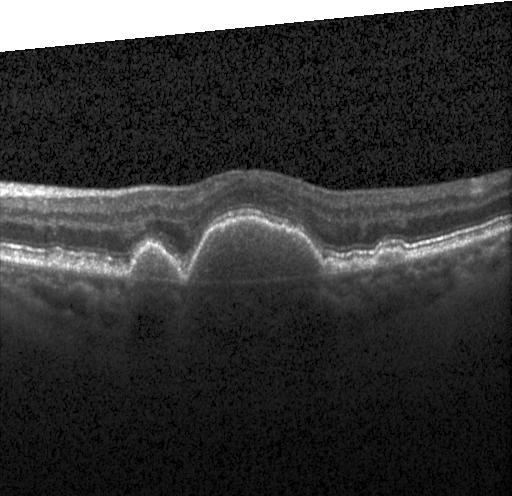
Optical coherence tomography B-scan. Heidelberg Spectralis OCT system. Impression: choroidal neovascularization.